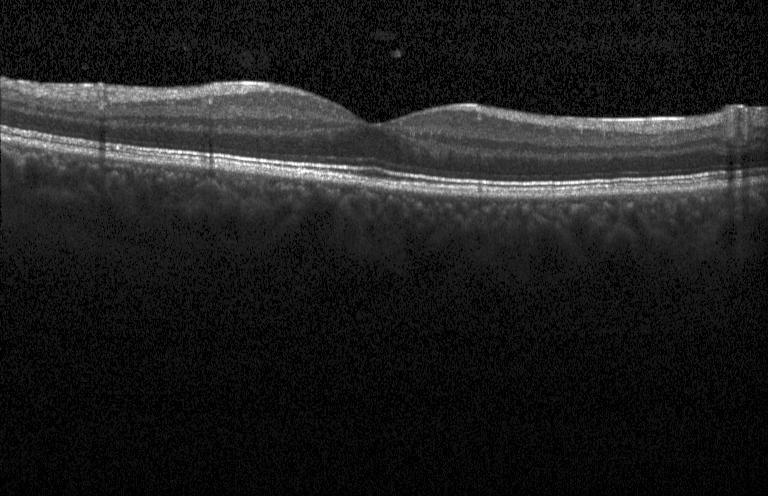
OCT scan showing no evidence of choroidal neovascularization, diabetic macular edema, or drusen.